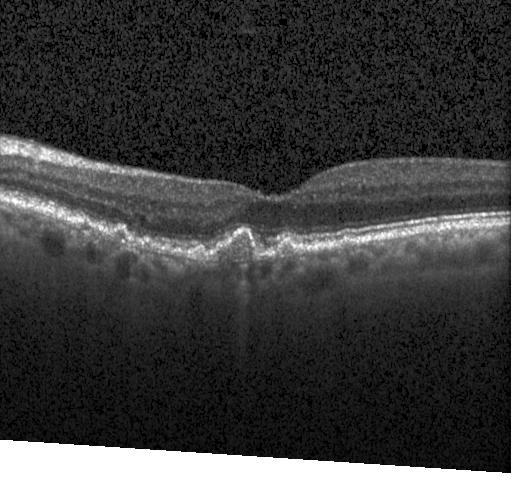 SD-OCT, retinal OCT B-scan, Heidelberg Spectralis, through the macula — Finding: sub-RPE drusenoid deposits.